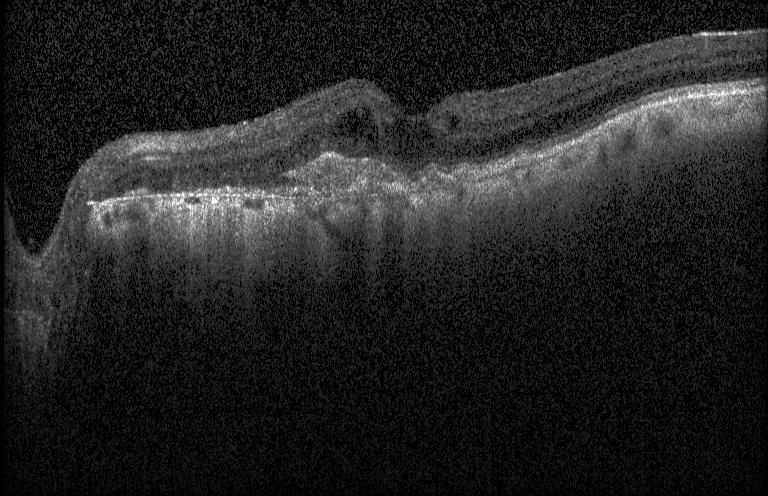
Optical coherence tomography B-scan — Finding: a choroidal neovascular membrane.